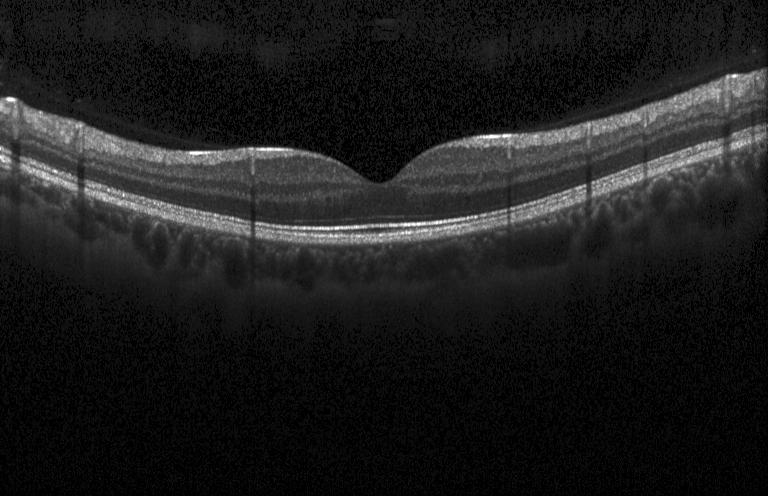
Fovea-centered. Retinal OCT B-scan.
This B-scan demonstrates neither CNV, DME, nor drusen.